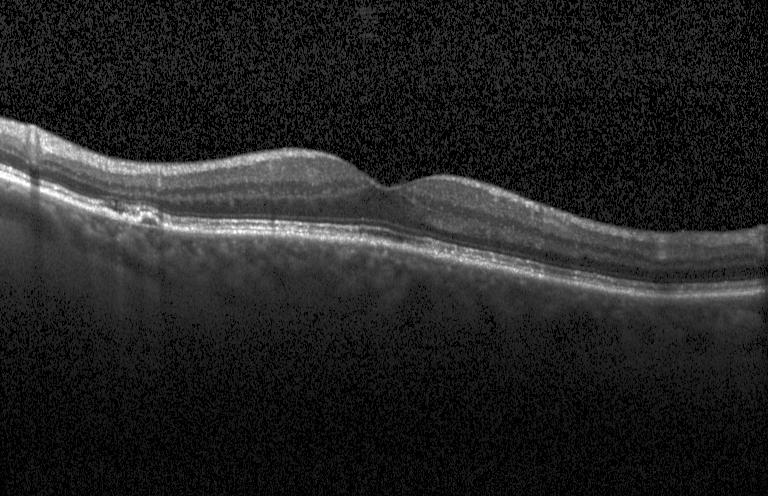 Impression: choroidal neovascularization.